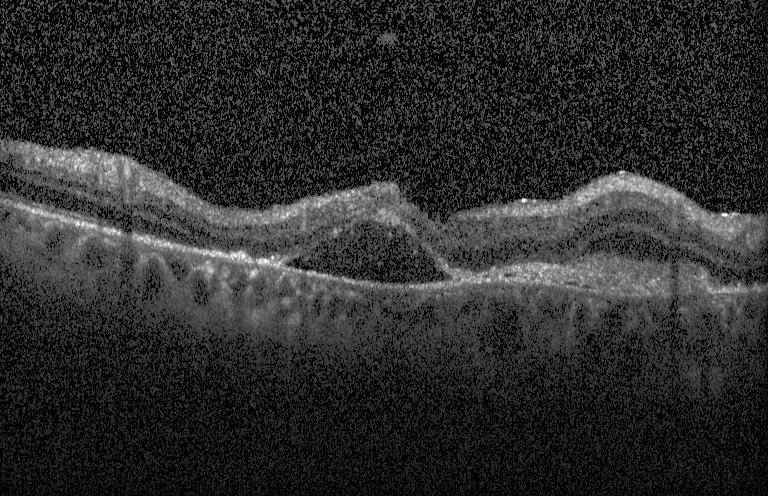

Spectral-domain OCT B-scan: choroidal neovascularization (CNV).